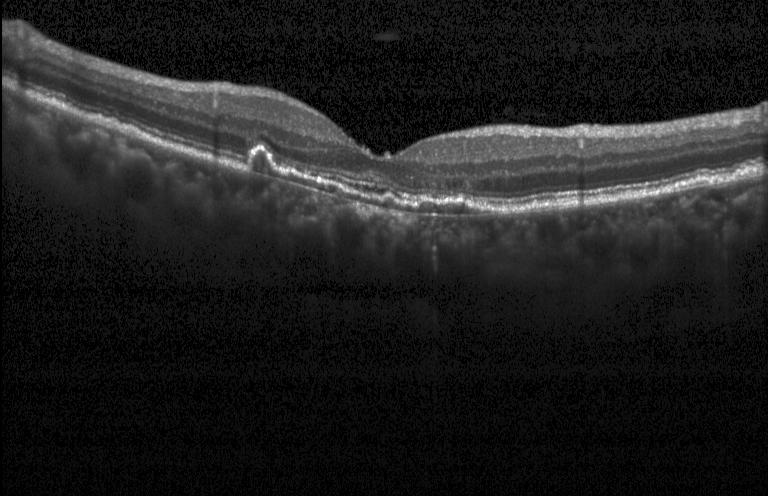 Heidelberg Spectralis OCT system. Through the macula. Optical coherence tomography scan — Finding: a choroidal neovascular membrane.